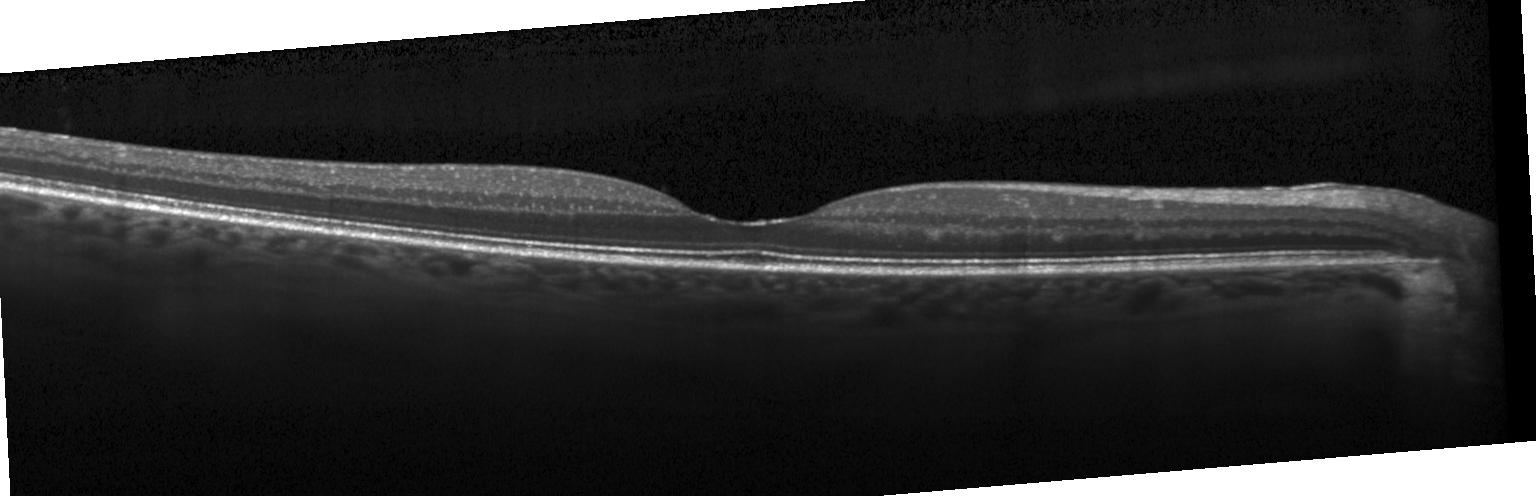
Finding: no CNV, DME, or drusen.